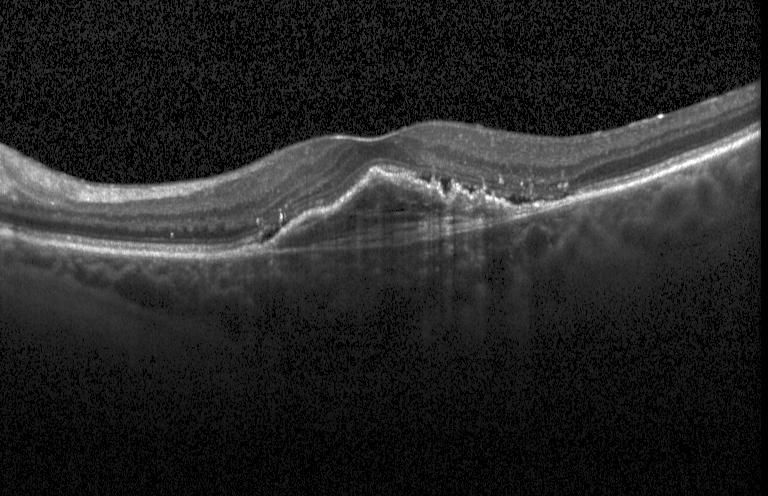
Finding: CNV.